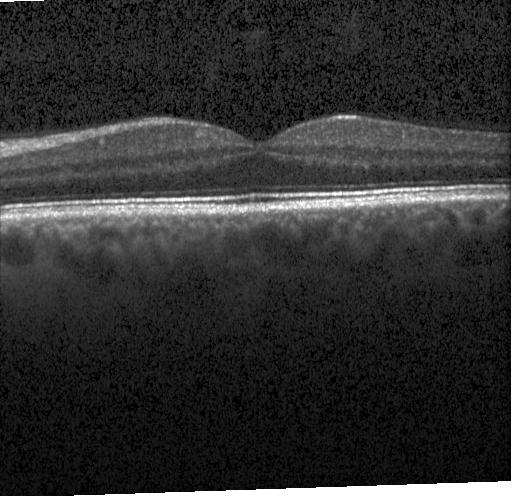 Optical coherence tomography B-scan; through the macula; spectral-domain optical coherence tomography; instrument: Heidelberg Spectralis — The scan shows neither CNV, DME, nor drusen.